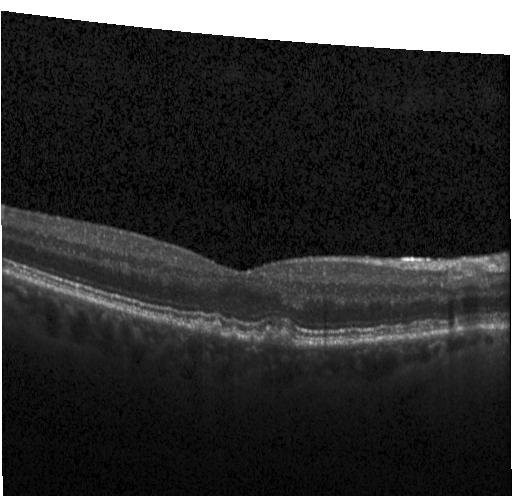

SD-OCT; optical coherence tomography B-scan; Heidelberg Spectralis OCT system
Finding: multiple drusen.